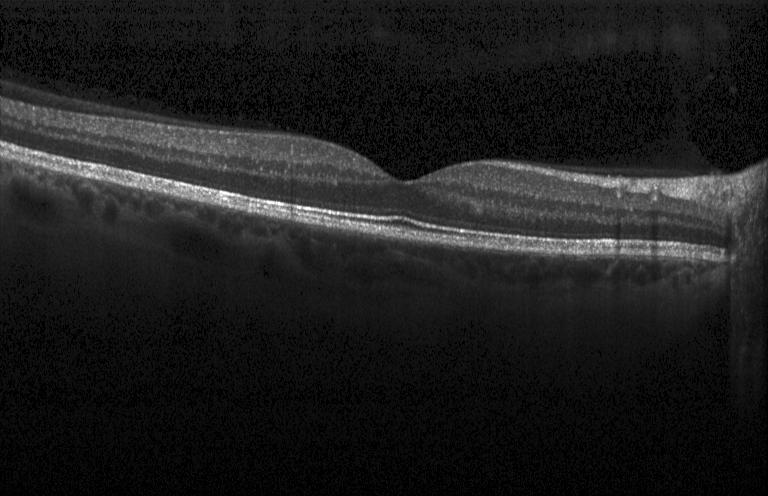

OCT line scan, spectral-domain optical coherence tomography. Finding: no CNV, DME, or drusen.